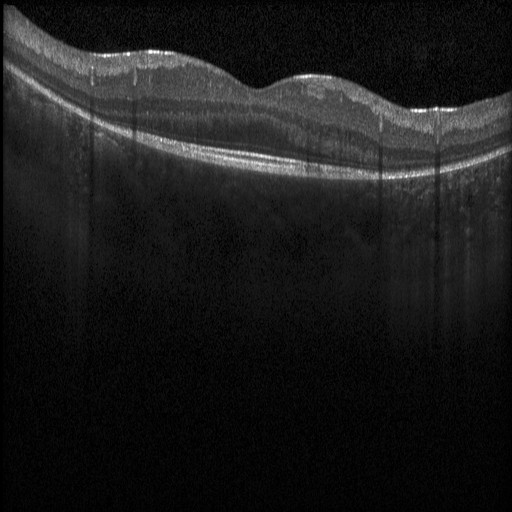

SD-OCT; macular scan; OCT B-scan.
Impression: DME.